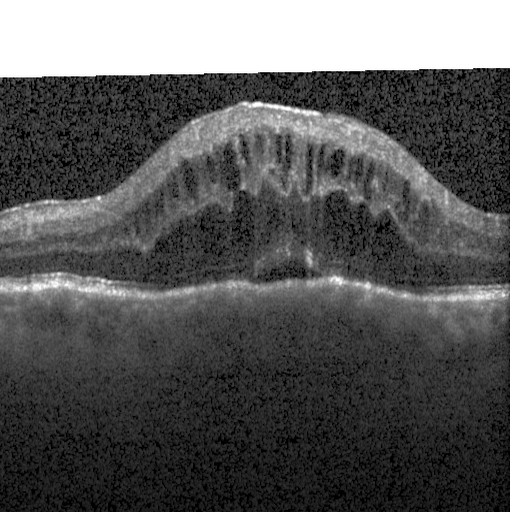

Heidelberg Spectralis; SD-OCT; retinal OCT cross-section; macular scan. Impression: diabetic macular edema (DME).